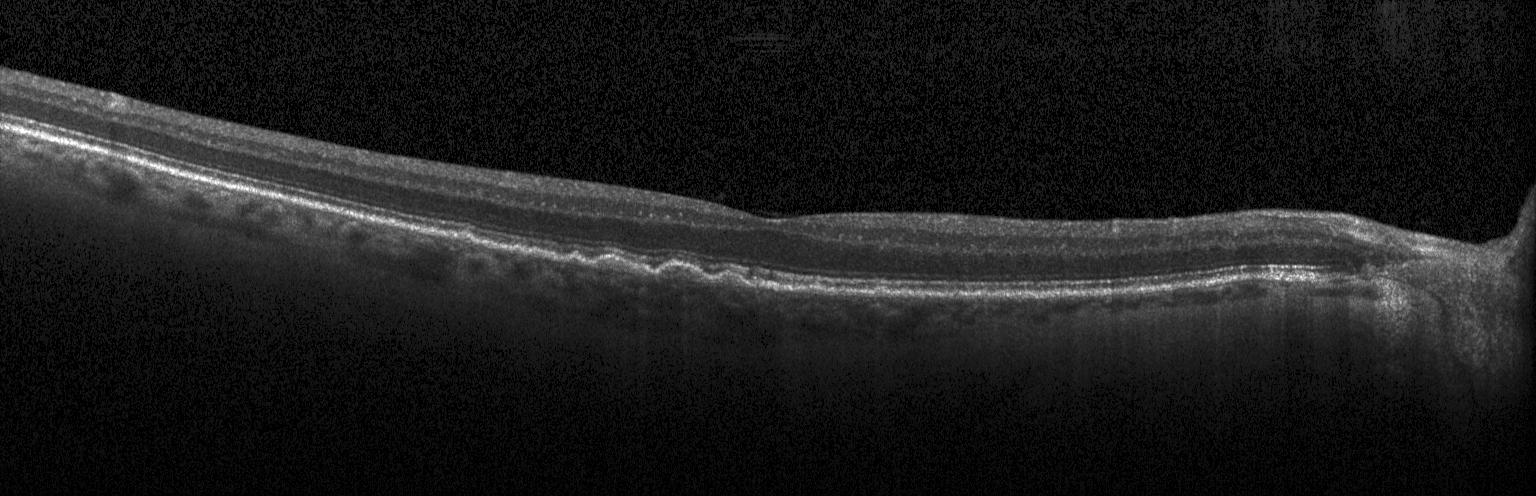

Optical coherence tomography B-scan.
Finding: drusen.